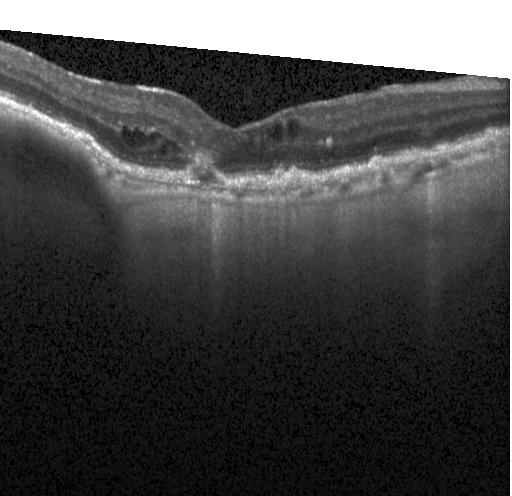

Diagnosis: a choroidal neovascular membrane.